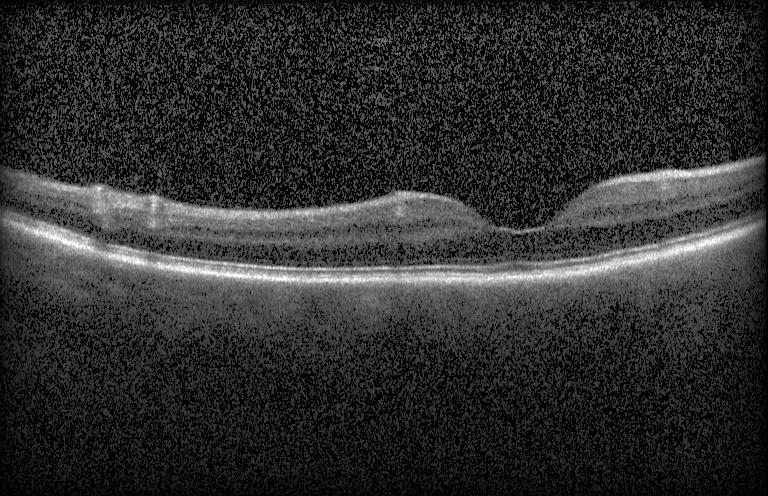

Spectral-domain OCT; fovea-centered; retinal OCT cross-section; Heidelberg Spectralis
Finding: no choroidal neovascularization, no diabetic macular edema, and no drusen.